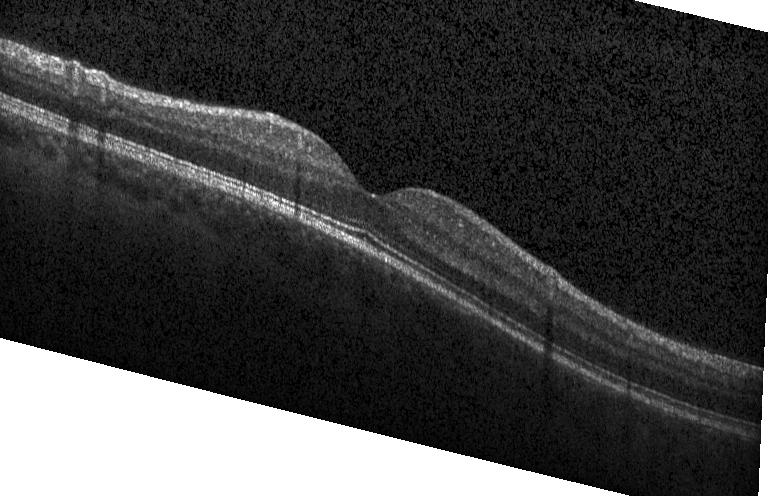 OCT line scan — The scan shows no CNV, DME, or drusen.